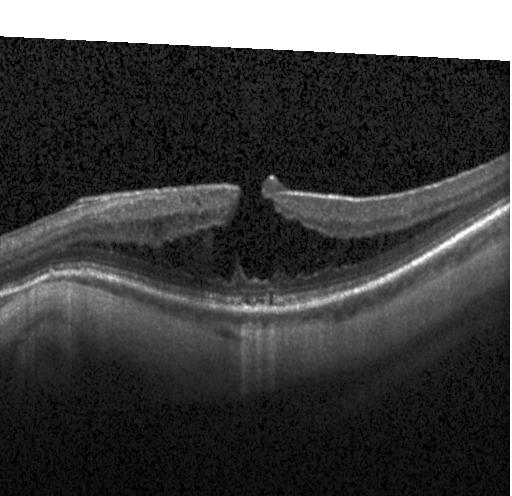
Macular OCT: diabetic macular edema.